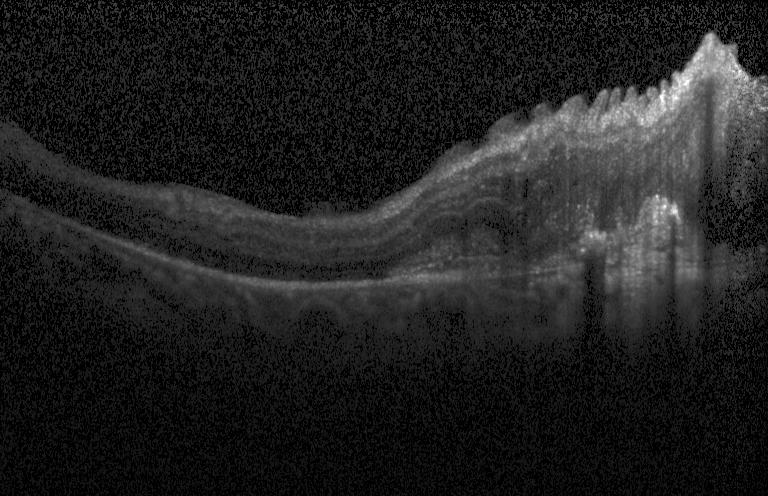
Spectral-domain optical coherence tomography, retinal OCT cross-section, macular scan.
Finding: CNV.